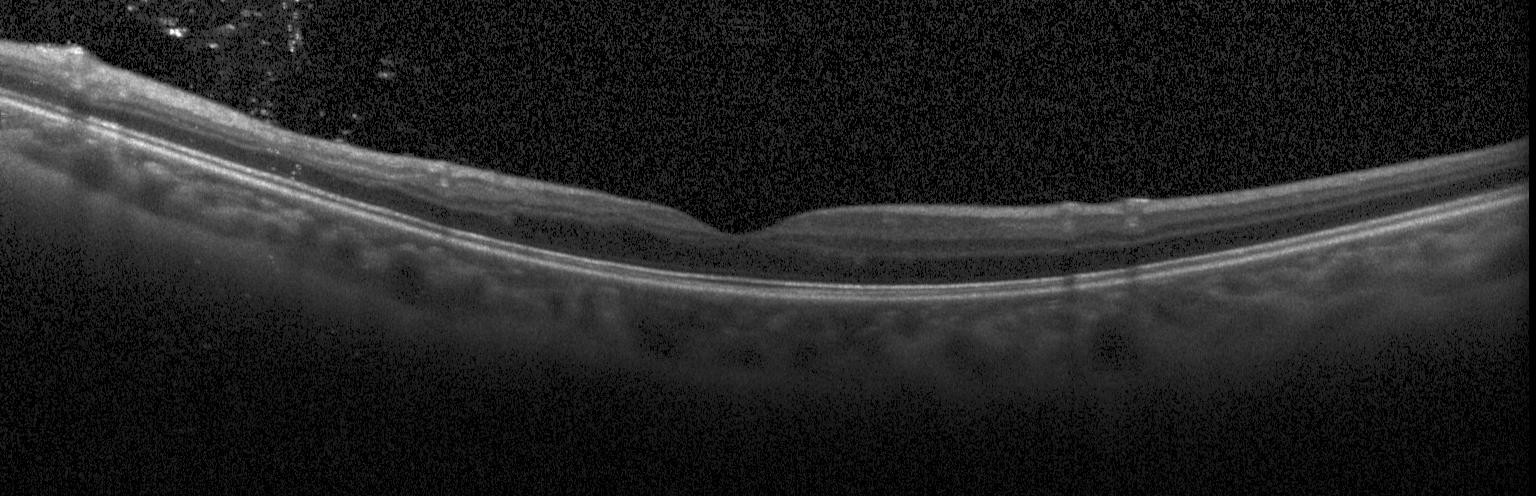 Spectral-domain OCT, retinal OCT cross-section, instrument: Heidelberg Spectralis.
Neither choroidal neovascularization, diabetic macular edema, nor drusen.